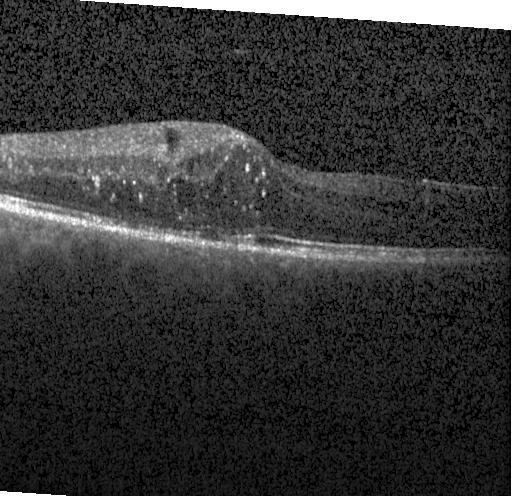
Diabetic macular edema (DME).